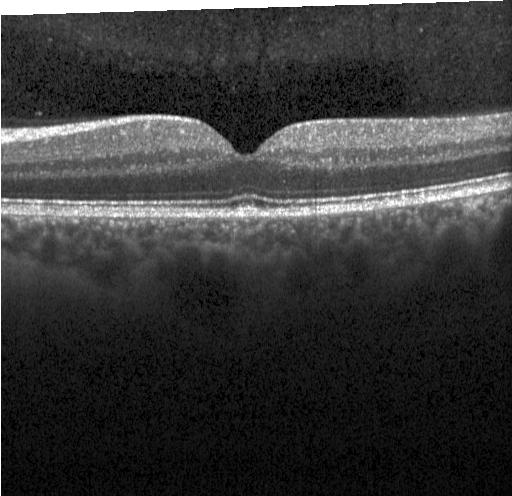

Instrument: Heidelberg Spectralis, optical coherence tomography scan, centered on the fovea, spectral-domain OCT.
Diagnosis: no CNV, DME, or drusen.